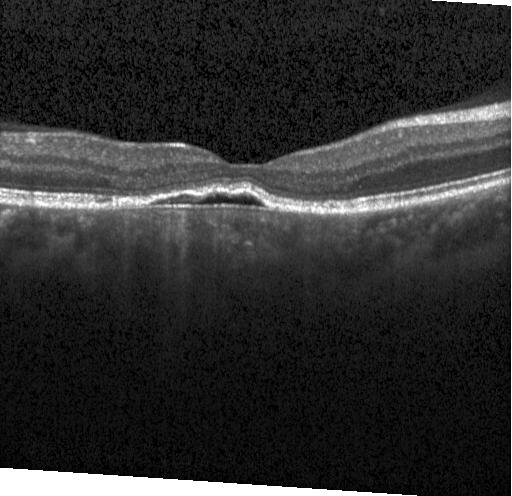 Horizontal scan through the fovea. Spectral-domain OCT. Acquired on a Heidelberg Spectralis. Optical coherence tomography B-scan — Finding: a choroidal neovascular membrane.